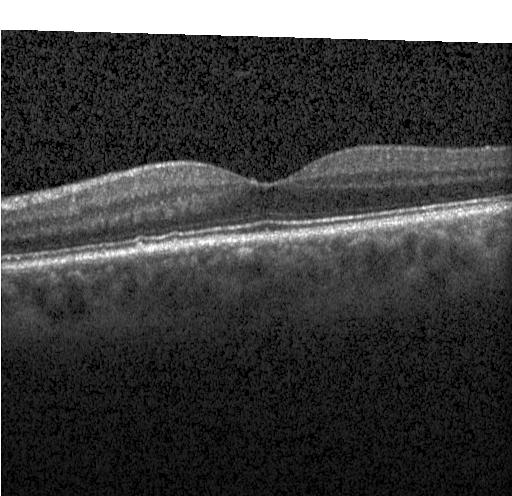
Optical coherence tomography B-scan — The scan shows multiple drusen.